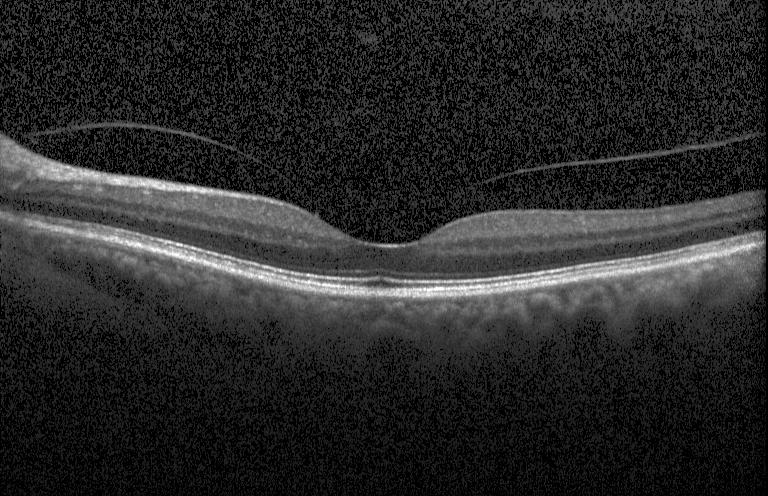

Optical coherence tomography B-scan — Finding: no choroidal neovascularization, diabetic macular edema, or drusen.